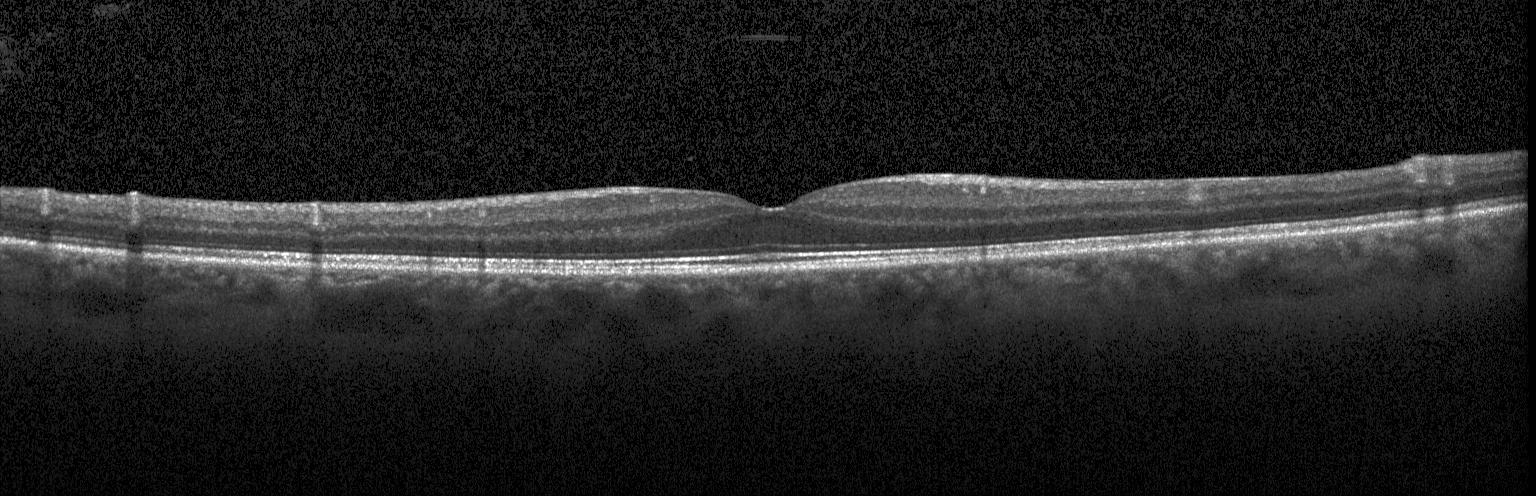
Diagnosis: no choroidal neovascularization, no diabetic macular edema, and no drusen.